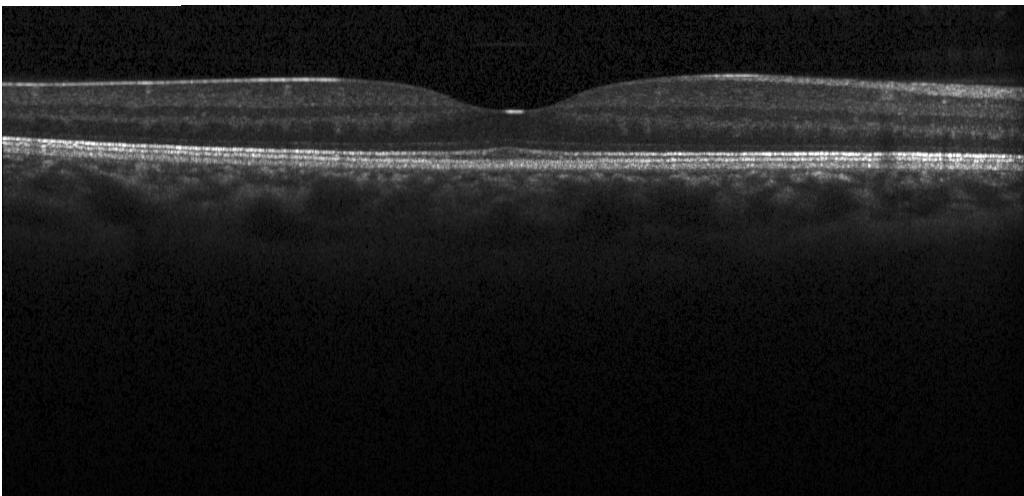
SD-OCT; instrument: Heidelberg Spectralis; optical coherence tomography scan
Finding: no choroidal neovascularization, diabetic macular edema, or drusen.